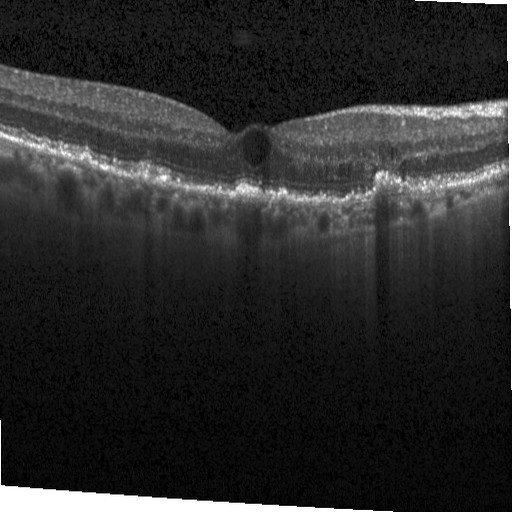
OCT finding: diabetic macular edema.